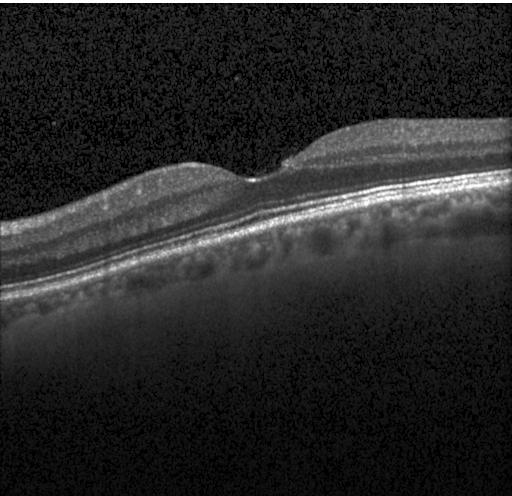 Instrument: Heidelberg Spectralis. SD-OCT. Macular scan. Optical coherence tomography B-scan. The scan shows no choroidal neovascularization, diabetic macular edema, or drusen.